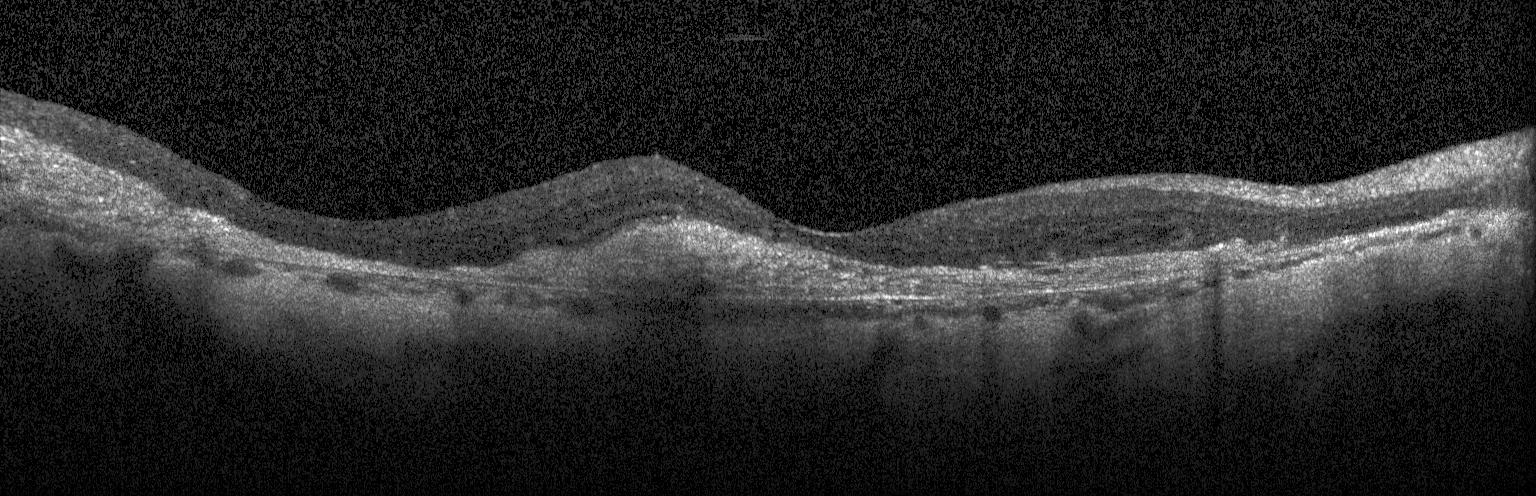 Acquired on a Heidelberg Spectralis; SD-OCT; retinal OCT B-scan; through the macula
Assessment: CNV.